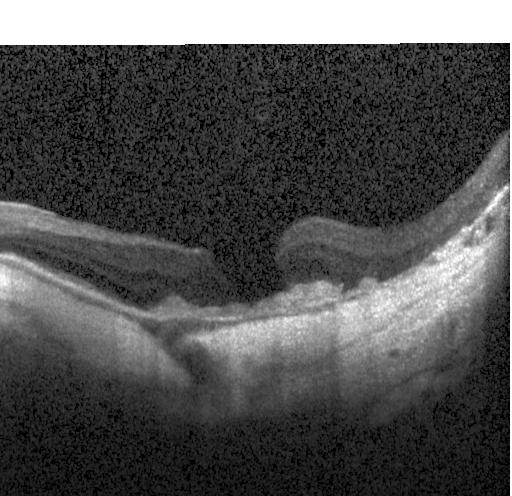

OCT line scan, spectral-domain OCT, instrument: Heidelberg Spectralis, fovea-centered
The scan shows a choroidal neovascular membrane.